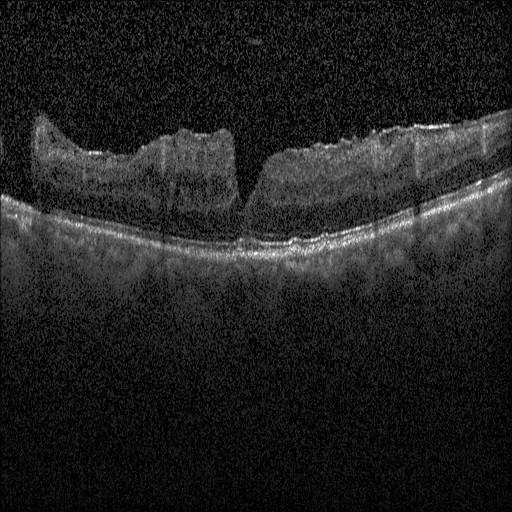

Heidelberg Spectralis, OCT B-scan, SD-OCT, macular scan
This B-scan demonstrates diabetic macular edema.